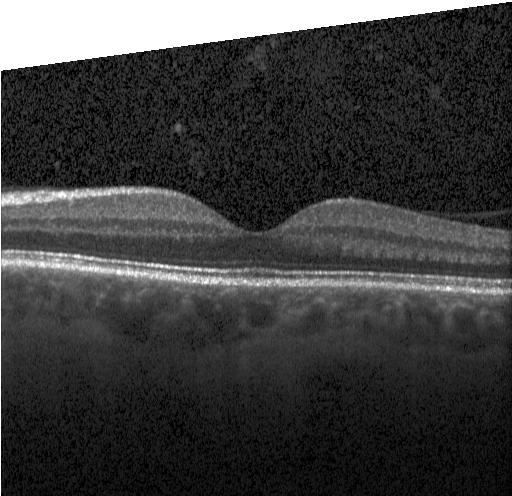

Optical coherence tomography B-scan. This B-scan demonstrates no CNV, DME, or drusen.